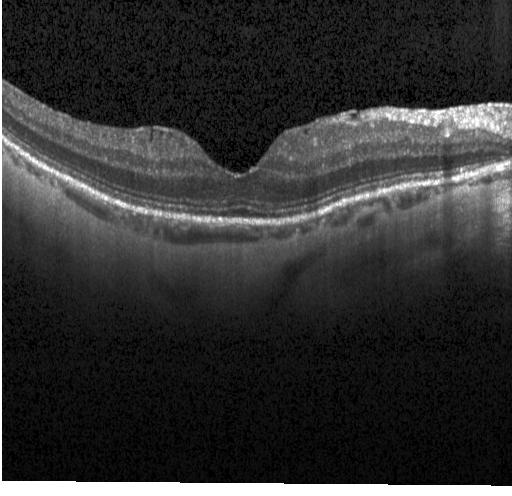
Macular OCT: no evidence of choroidal neovascularization, diabetic macular edema, or drusen.